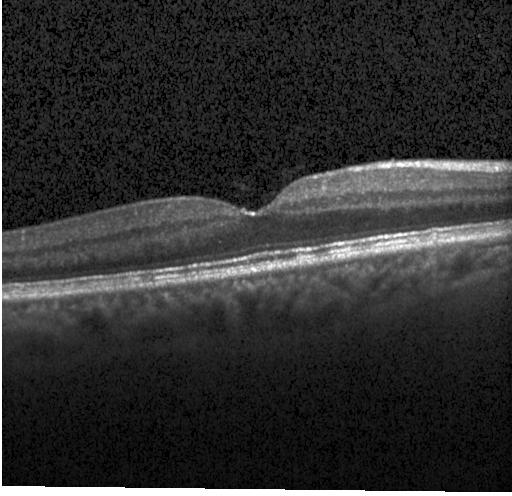
OCT line scan. Macular scan — This B-scan demonstrates no choroidal neovascularization, diabetic macular edema, or drusen.